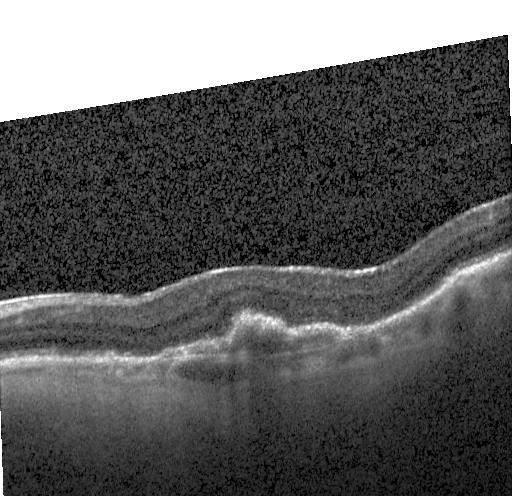

OCT B-scan showing choroidal neovascularization.